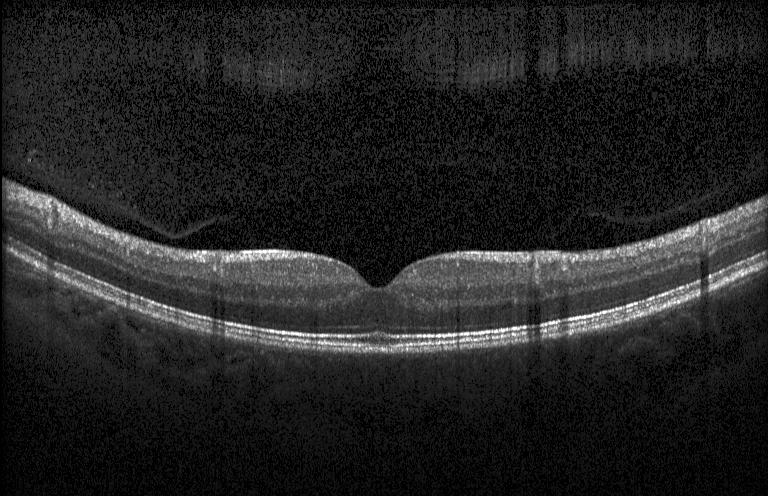
Heidelberg Spectralis OCT system, OCT B-scan
Finding: neither choroidal neovascularization, diabetic macular edema, nor drusen.